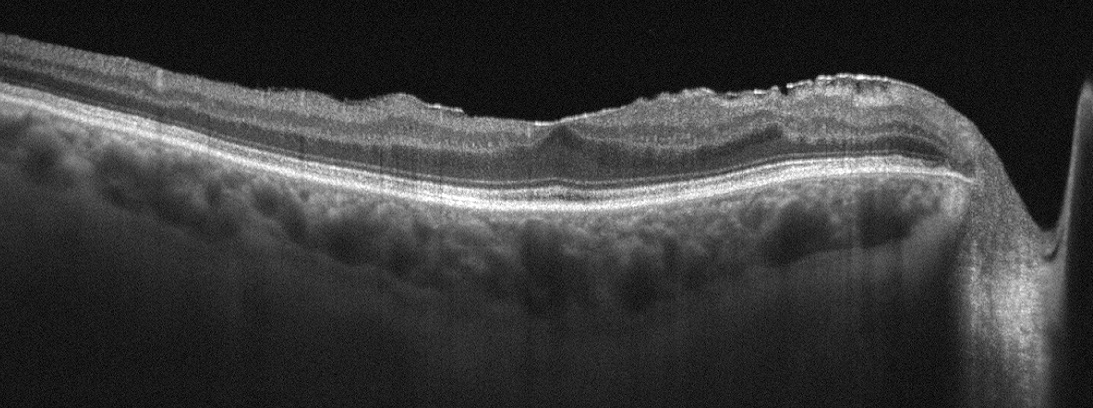

OCT B-scan. Diagnosis: epiretinal membrane (ERM).